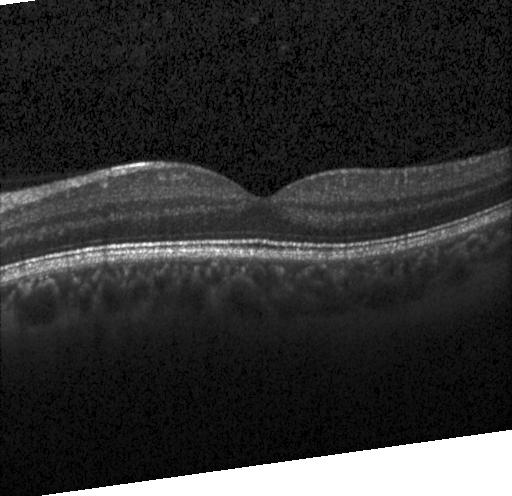
OCT line scan
Finding: no evidence of CNV, DME, or drusen.